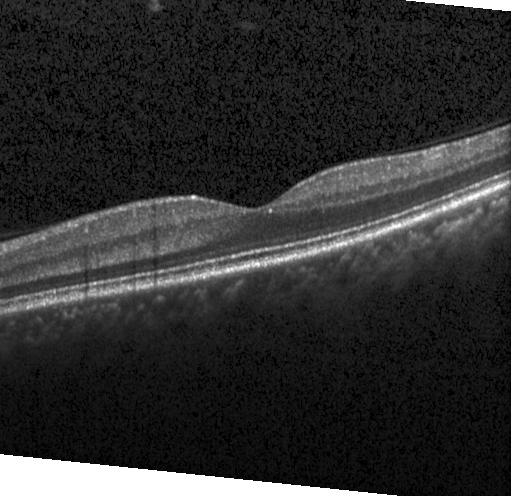

OCT line scan
Impression: no choroidal neovascularization, no diabetic macular edema, and no drusen.